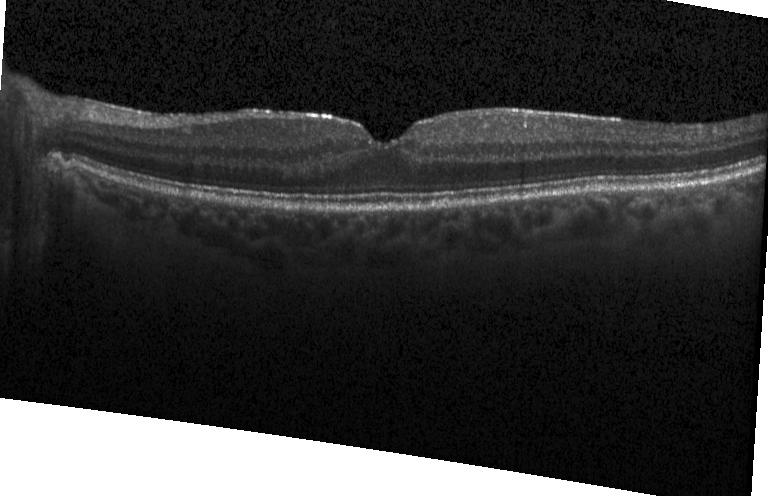 Through the macula · Heidelberg Spectralis OCT system · spectral-domain optical coherence tomography · OCT B-scan — OCT finding: neither choroidal neovascularization, diabetic macular edema, nor drusen.